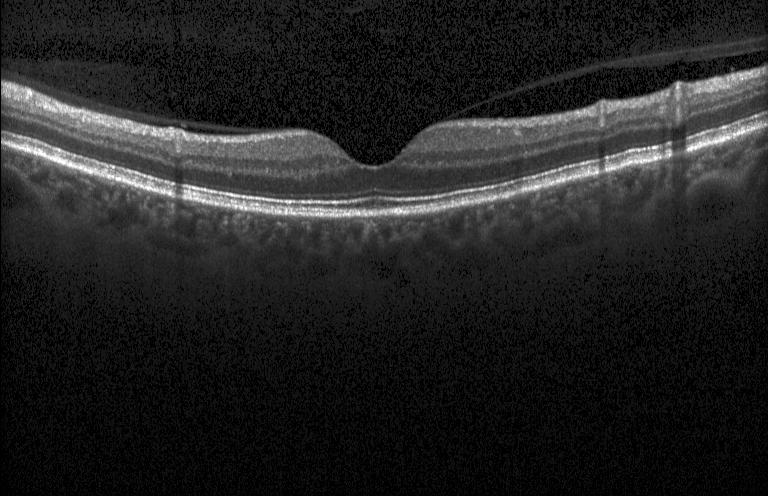
SD-OCT · horizontal scan through the fovea · acquired on a Heidelberg Spectralis · optical coherence tomography scan.
This B-scan demonstrates no evidence of CNV, DME, or drusen.